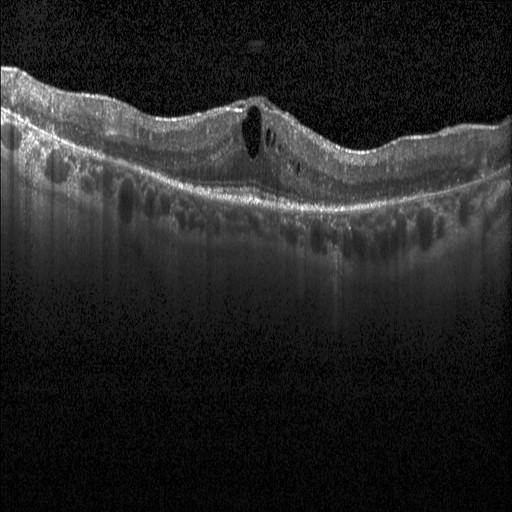
Retinal OCT cross-section, fovea-centered, spectral-domain optical coherence tomography.
Finding: DME.